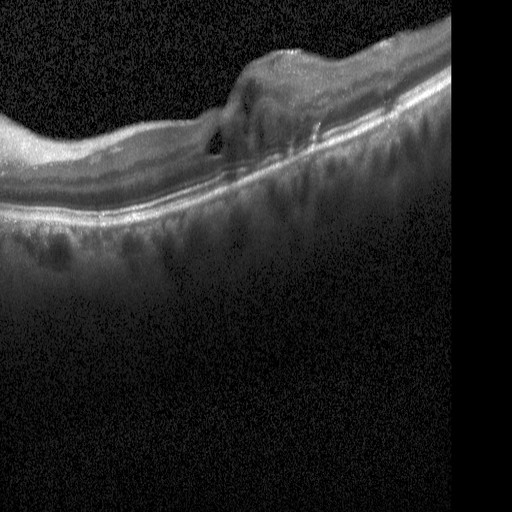 Through the macula · Heidelberg Spectralis OCT system · SD-OCT · optical coherence tomography B-scan.
The scan shows DME.